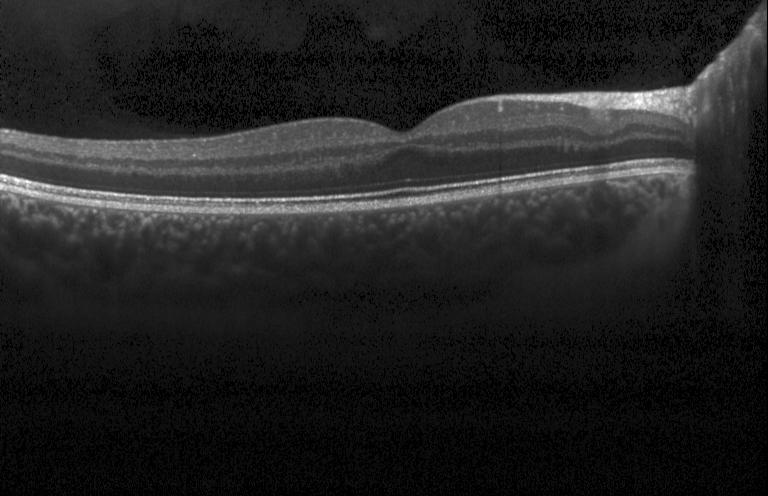 OCT B-scan · SD-OCT · instrument: Heidelberg Spectralis.
Finding: no evidence of CNV, DME, or drusen.